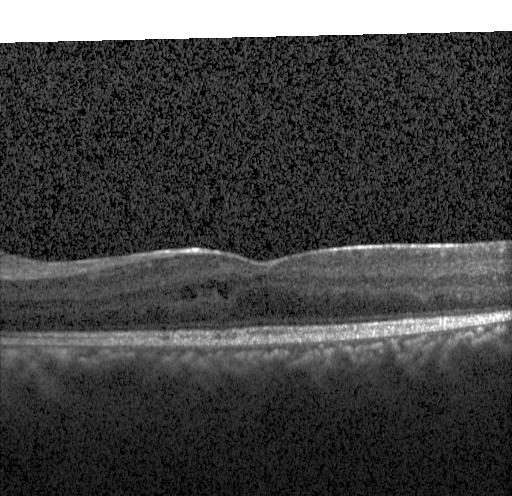
Optical coherence tomography scan, centered on the fovea, SD-OCT — Impression: DME.